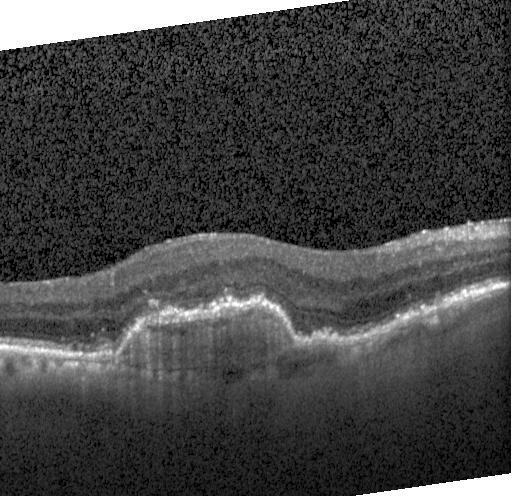 Impression: choroidal neovascularization.